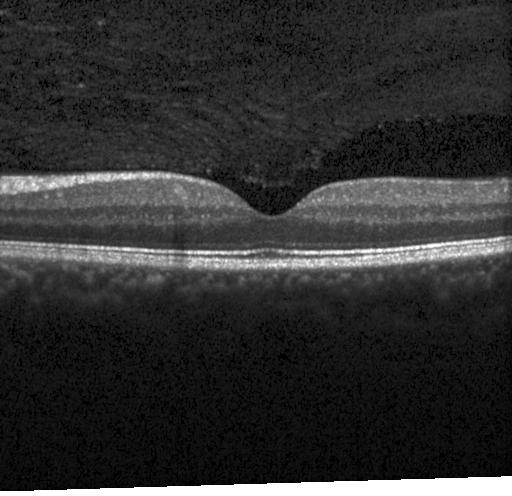
Instrument: Heidelberg Spectralis. Optical coherence tomography scan. SD-OCT. Through the macula.
This B-scan demonstrates neither choroidal neovascularization, diabetic macular edema, nor drusen.